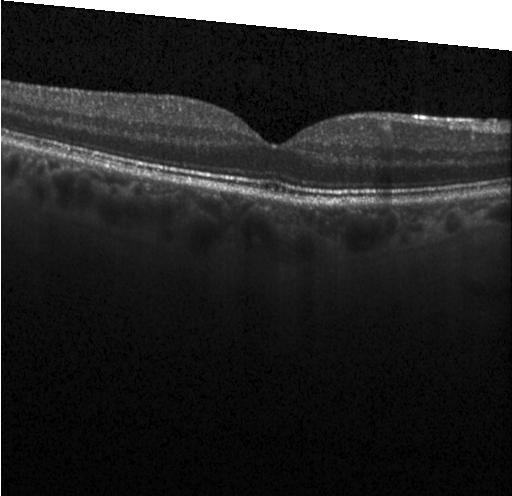

The scan shows no CNV, DME, or drusen.